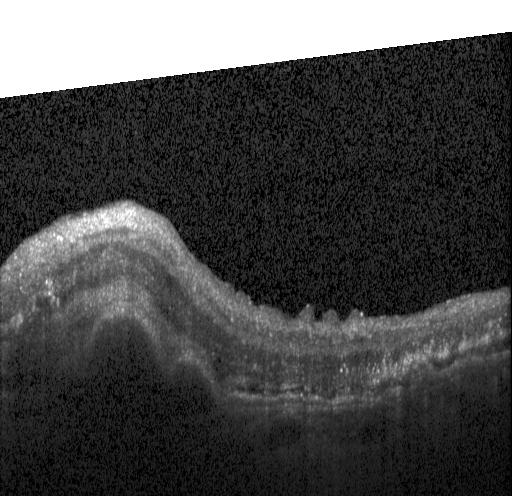

Macular OCT: choroidal neovascularization (CNV).